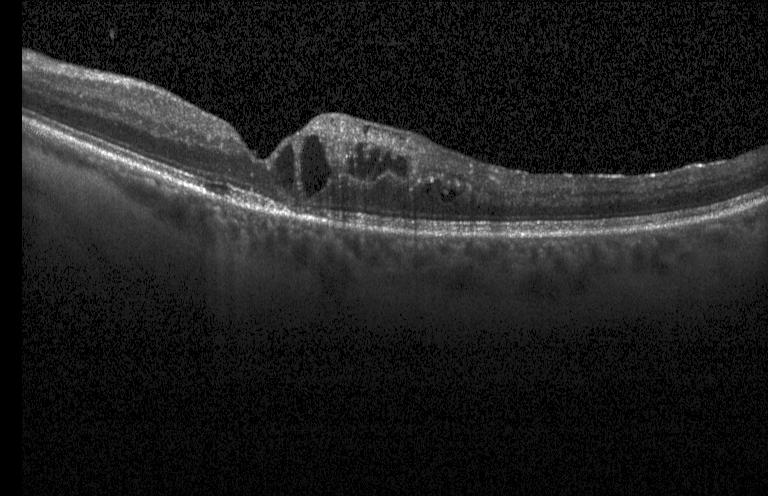
Retinal OCT cross-section. Spectral-domain optical coherence tomography. Instrument: Heidelberg Spectralis
Dx: diabetic macular edema.